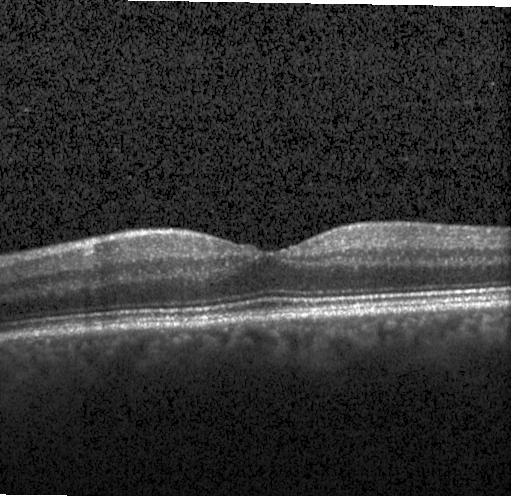
SD-OCT · Heidelberg Spectralis OCT system · OCT B-scan — Macular OCT: no evidence of choroidal neovascularization, diabetic macular edema, or drusen.